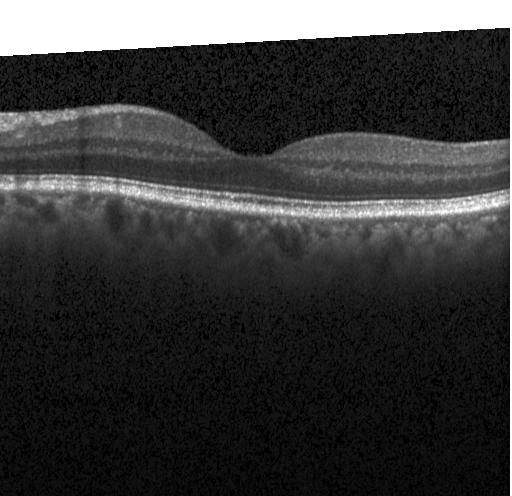 Optical coherence tomography scan — OCT finding: no evidence of choroidal neovascularization, diabetic macular edema, or drusen.